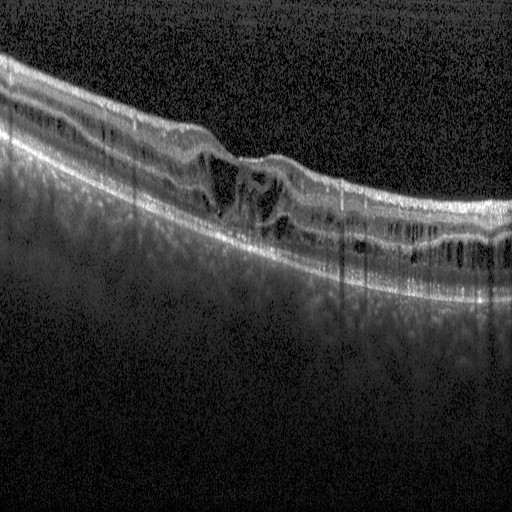 Through the macula. Instrument: Heidelberg Spectralis. OCT B-scan. Spectral-domain OCT. This B-scan demonstrates diabetic macular edema (DME).